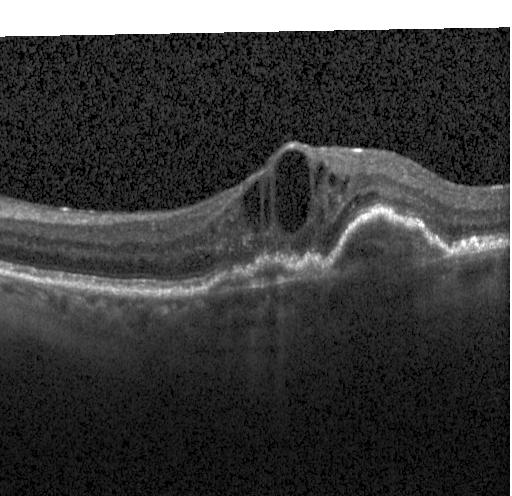

OCT B-scan · fovea-centered.
This B-scan demonstrates choroidal neovascularization.